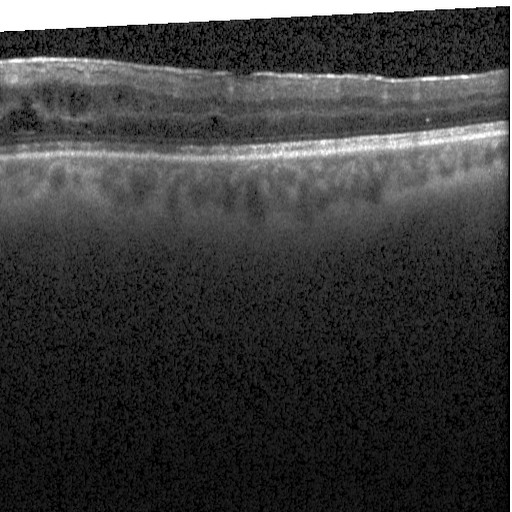
Diabetic macular edema.